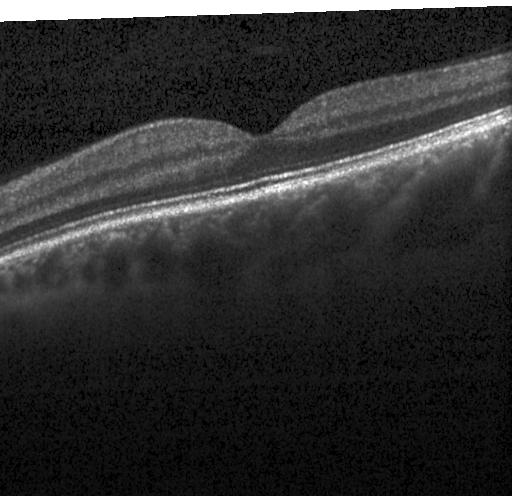 OCT B-scan showing no CNV, DME, or drusen.